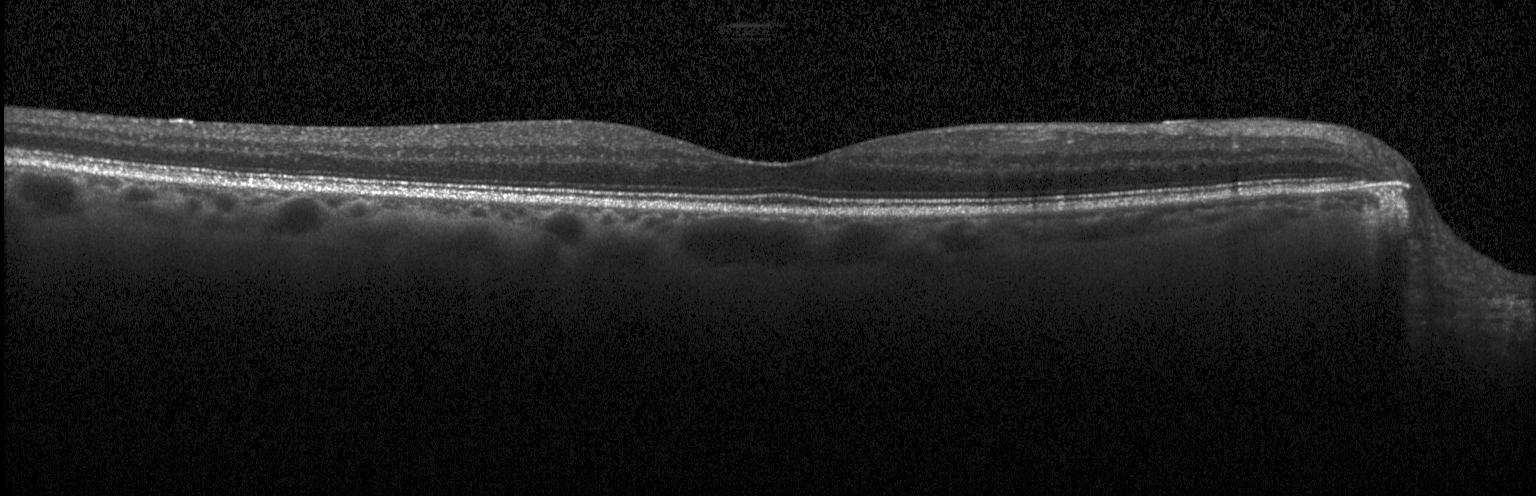
Optical coherence tomography scan. This B-scan demonstrates no choroidal neovascularization, diabetic macular edema, or drusen.